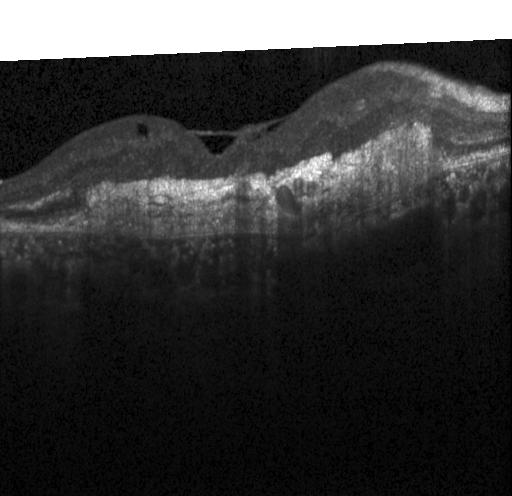

Retinal OCT B-scan; SD-OCT; horizontal scan through the fovea — Macular OCT: a choroidal neovascular membrane.